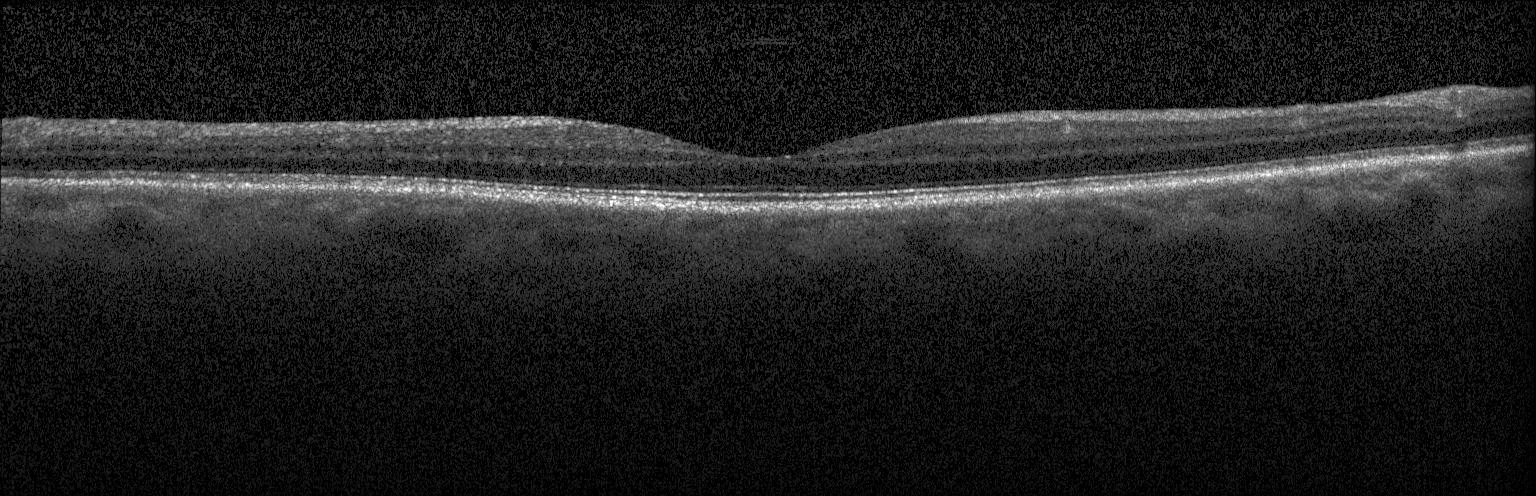
Instrument: Heidelberg Spectralis; optical coherence tomography B-scan; centered on the fovea. Finding: no choroidal neovascularization, no diabetic macular edema, and no drusen.